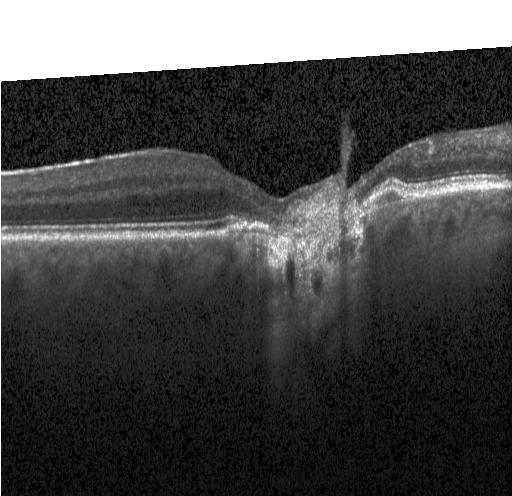

Through the macula; OCT B-scan; spectral-domain OCT. Impression: choroidal neovascularization (CNV).